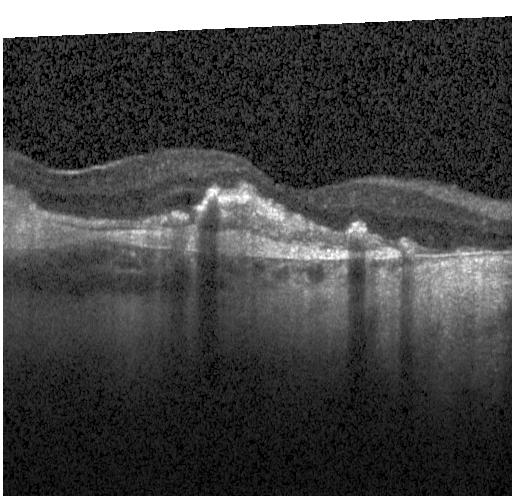 Diagnosis: a choroidal neovascular membrane.